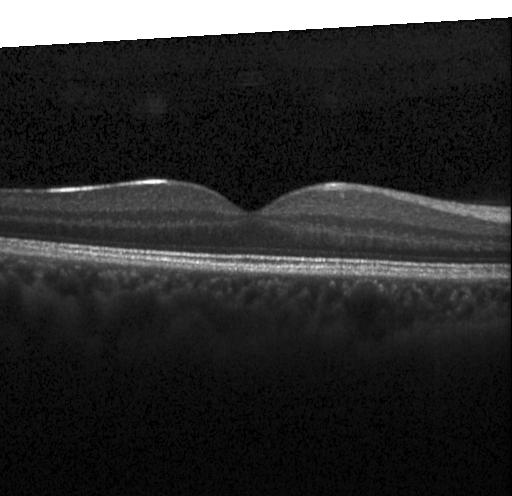 SD-OCT; retinal OCT B-scan.
This B-scan demonstrates no evidence of CNV, DME, or drusen.